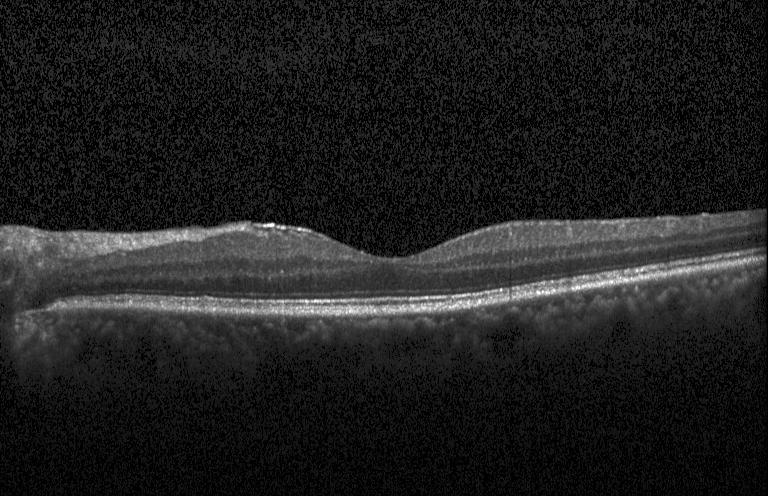

OCT finding: no evidence of choroidal neovascularization, diabetic macular edema, or drusen.